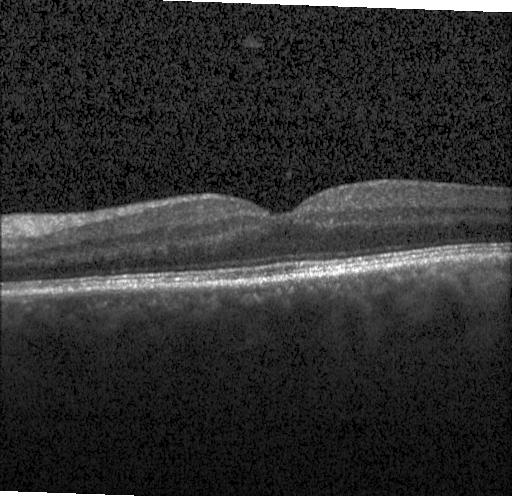
Retinal OCT B-scan.
Impression: neither choroidal neovascularization, diabetic macular edema, nor drusen.